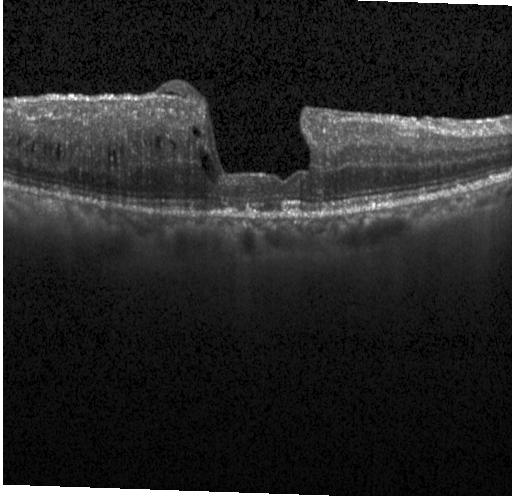
OCT line scan · centered on the fovea — Finding: diabetic macular edema.